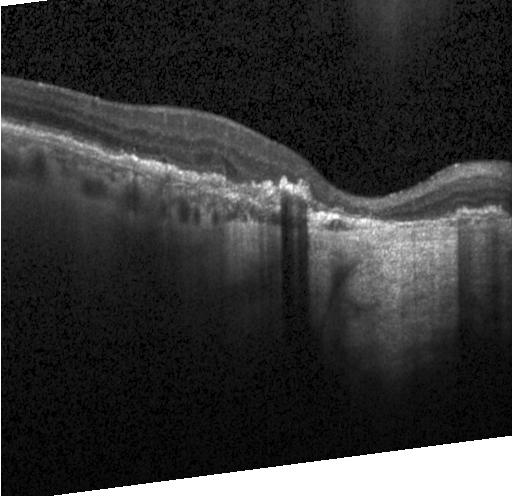 OCT finding: a choroidal neovascular membrane.